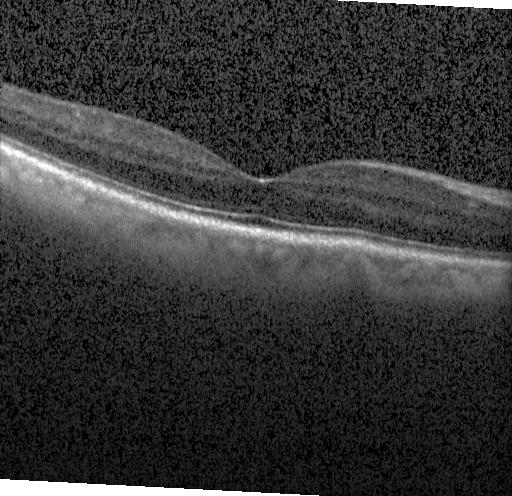 SD-OCT. Fovea-centered. Retinal OCT B-scan. Heidelberg Spectralis
Finding: no choroidal neovascularization, diabetic macular edema, or drusen.